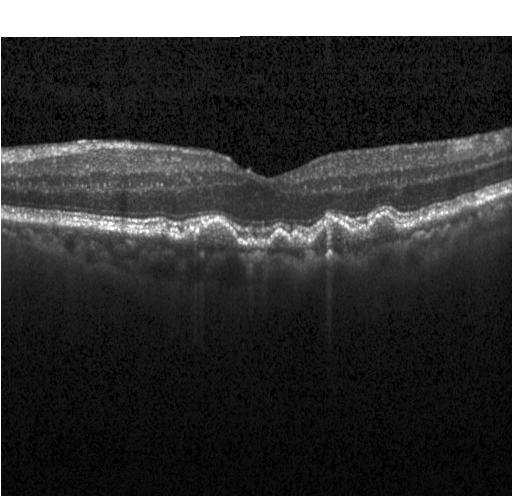
OCT line scan. Spectral-domain OCT. Through the macula. Instrument: Heidelberg Spectralis. Impression: drusen.